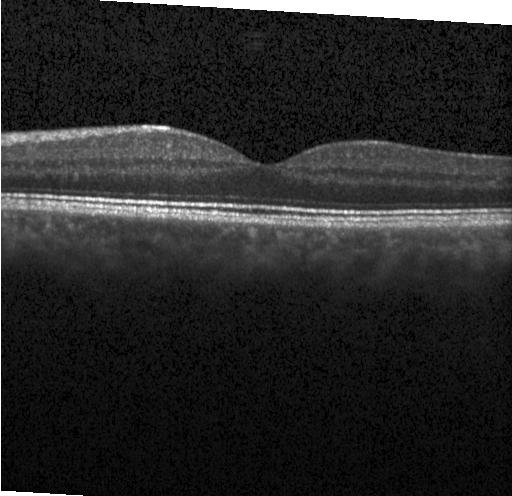
Spectral-domain optical coherence tomography; horizontal scan through the fovea; retinal OCT cross-section
Finding: no CNV, DME, or drusen.